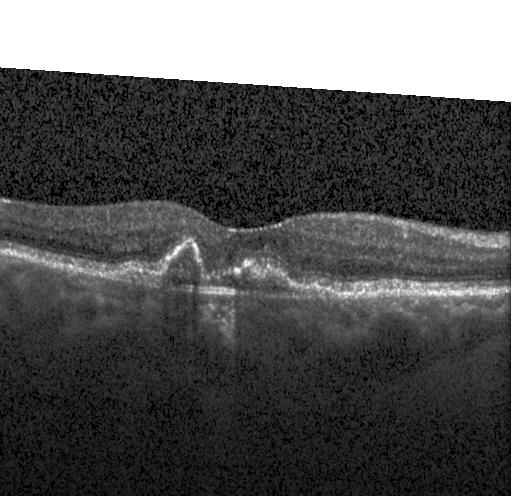

Optical coherence tomography scan; through the macula; instrument: Heidelberg Spectralis; spectral-domain OCT — CNV.